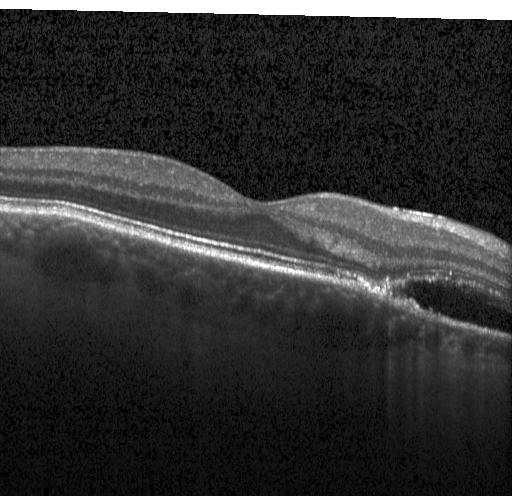
OCT B-scan.
Diagnosis: choroidal neovascularization.